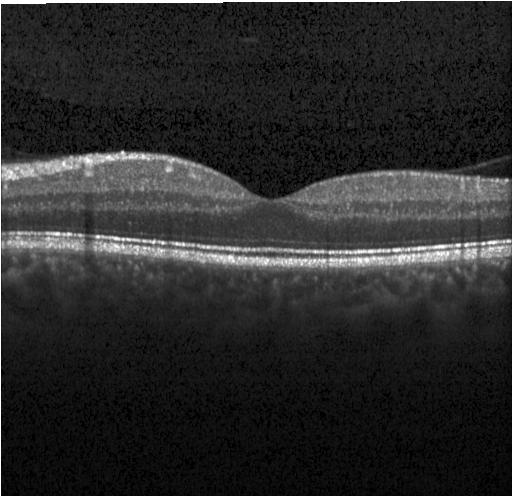 Dx: no choroidal neovascularization, diabetic macular edema, or drusen.